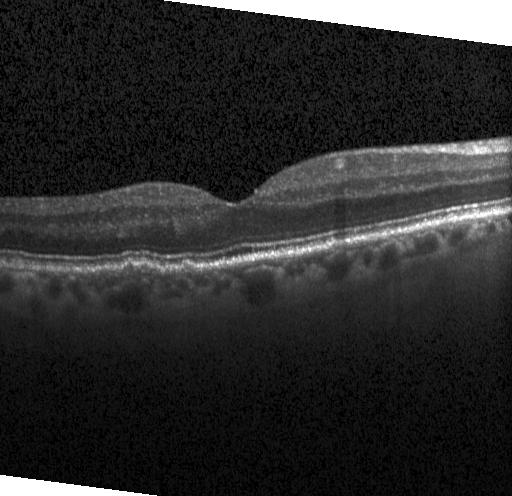 Horizontal scan through the fovea · Heidelberg Spectralis OCT system · OCT line scan · spectral-domain OCT — Diagnosis: multiple drusen.